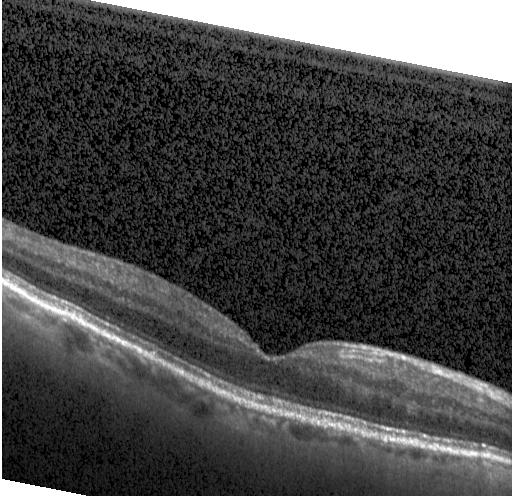 OCT line scan. Impression: no evidence of choroidal neovascularization, diabetic macular edema, or drusen.